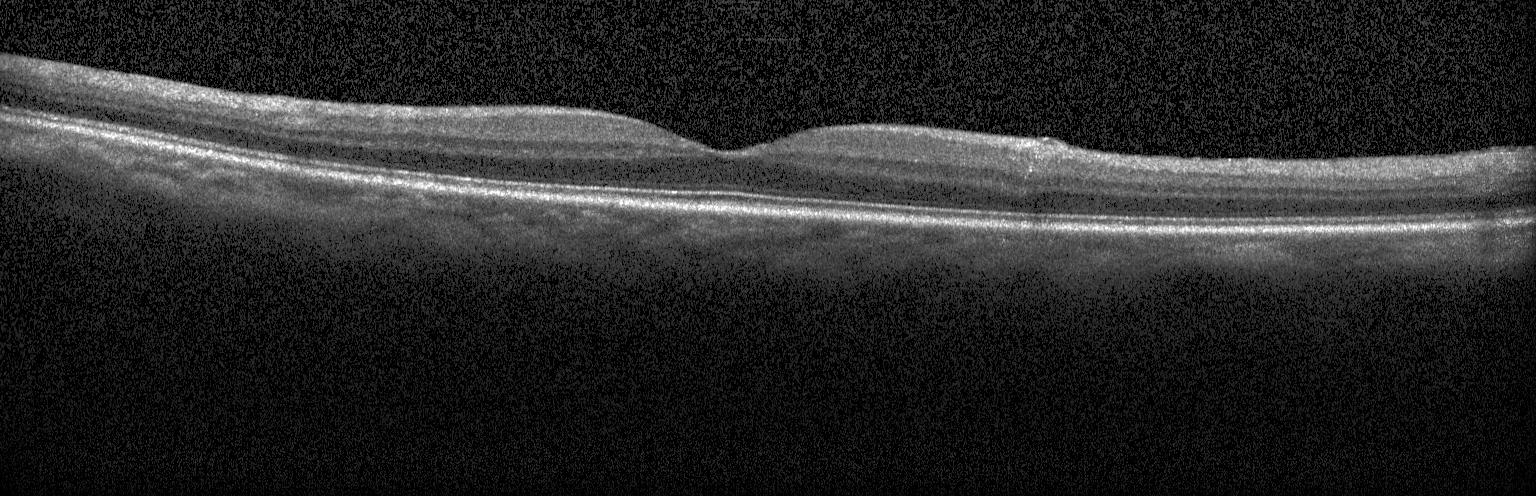 Finding: neither choroidal neovascularization, diabetic macular edema, nor drusen.